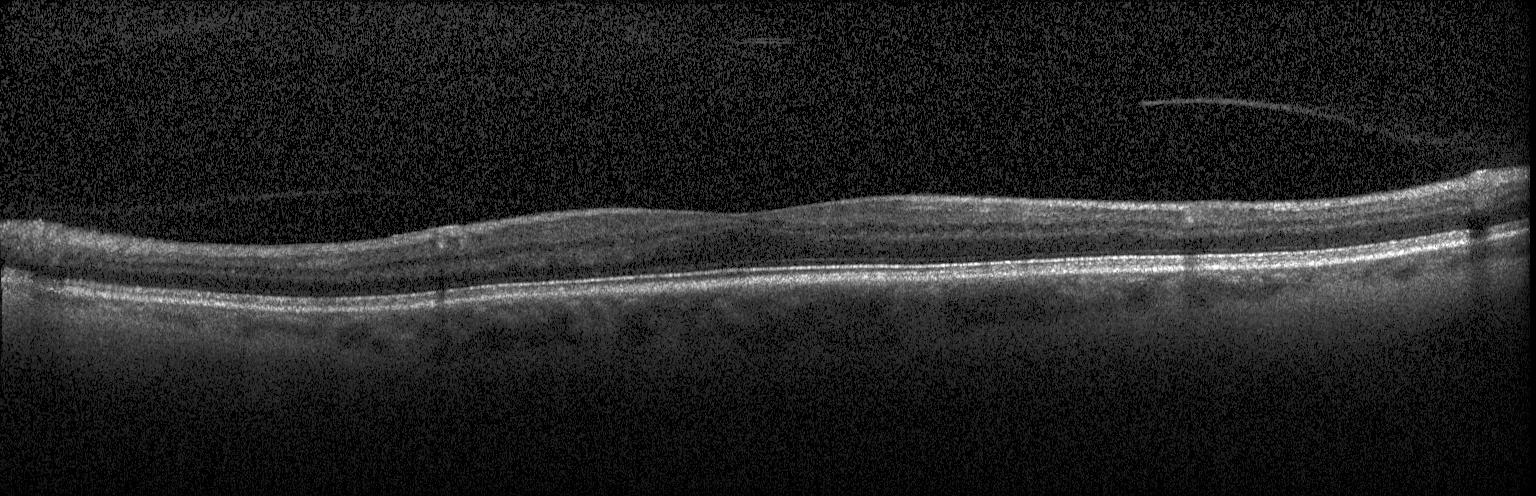
SD-OCT. Horizontal scan through the fovea. OCT B-scan
Diagnosis: no choroidal neovascularization, no diabetic macular edema, and no drusen.